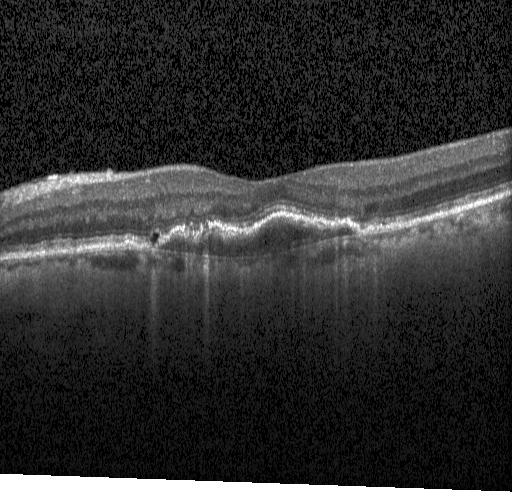
Fovea-centered, optical coherence tomography B-scan, Heidelberg Spectralis OCT system, spectral-domain OCT — Impression: choroidal neovascularization.